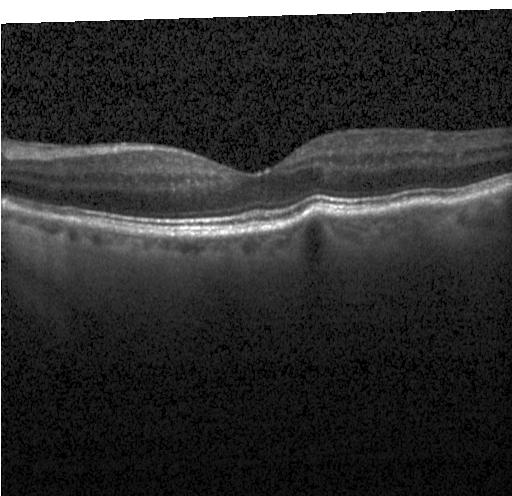
Centered on the fovea · SD-OCT · optical coherence tomography B-scan — Macular OCT: sub-RPE drusenoid deposits.